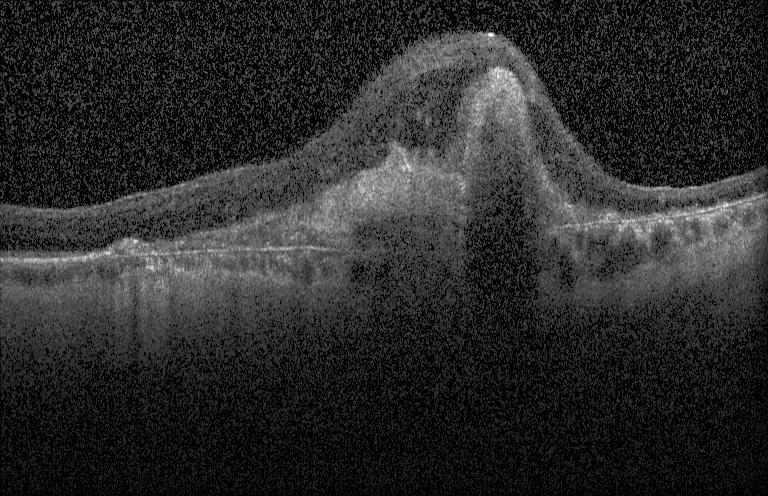

OCT B-scan, Heidelberg Spectralis, spectral-domain optical coherence tomography, through the macula — This B-scan demonstrates a choroidal neovascular membrane.